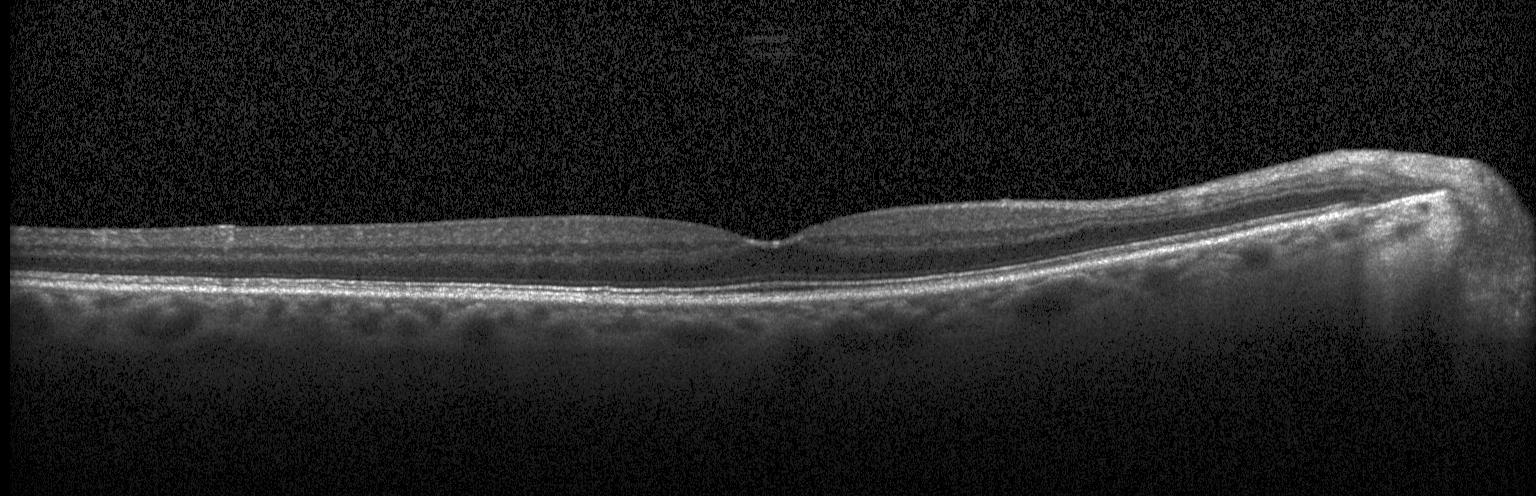
Acquired on a Heidelberg Spectralis; fovea-centered; retinal OCT cross-section; SD-OCT.
The scan shows no choroidal neovascularization, diabetic macular edema, or drusen.